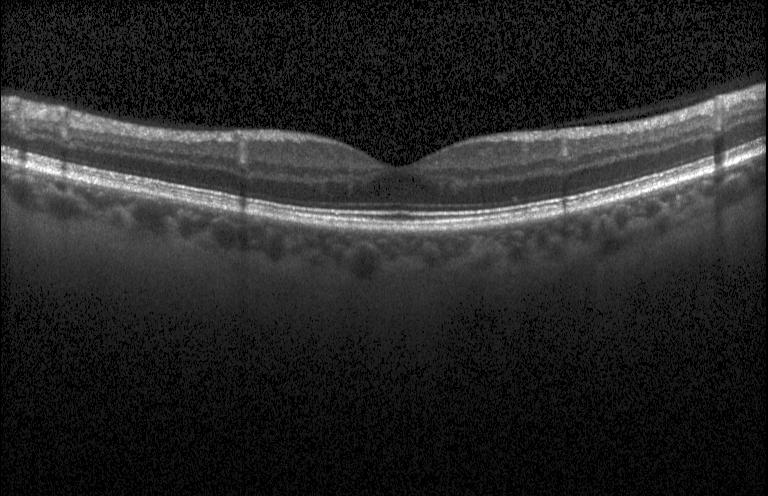 This B-scan demonstrates no CNV, DME, or drusen.